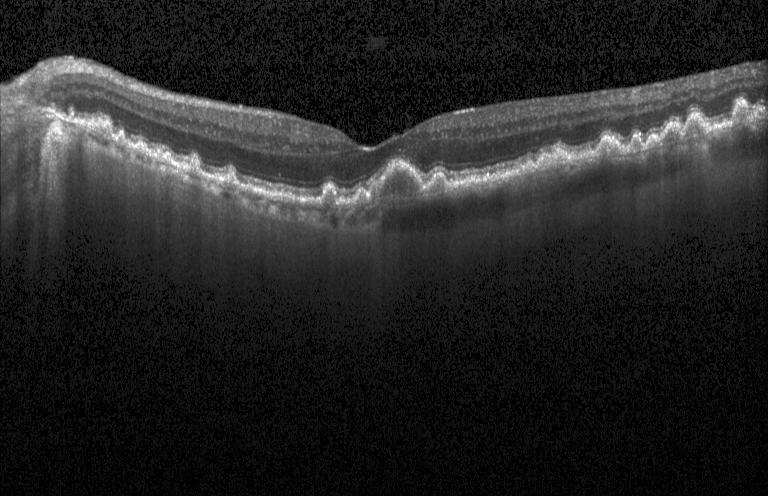

OCT B-scan. Centered on the fovea. Instrument: Heidelberg Spectralis — Finding: sub-RPE drusenoid deposits.